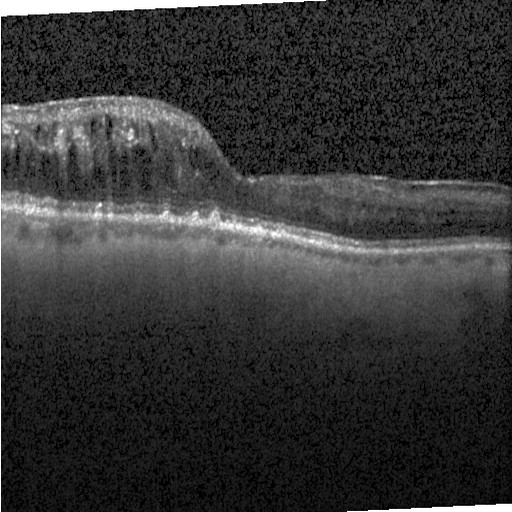
Macular scan; retinal OCT B-scan; instrument: Heidelberg Spectralis
Impression: diabetic macular edema.